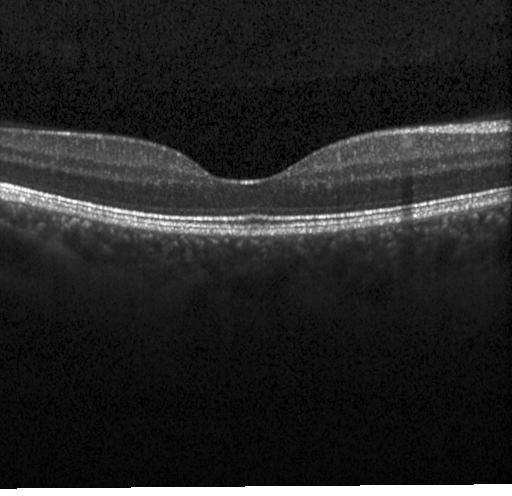

Horizontal scan through the fovea; spectral-domain OCT; retinal OCT cross-section — Diagnosis: no CNV, no DME, and no drusen.